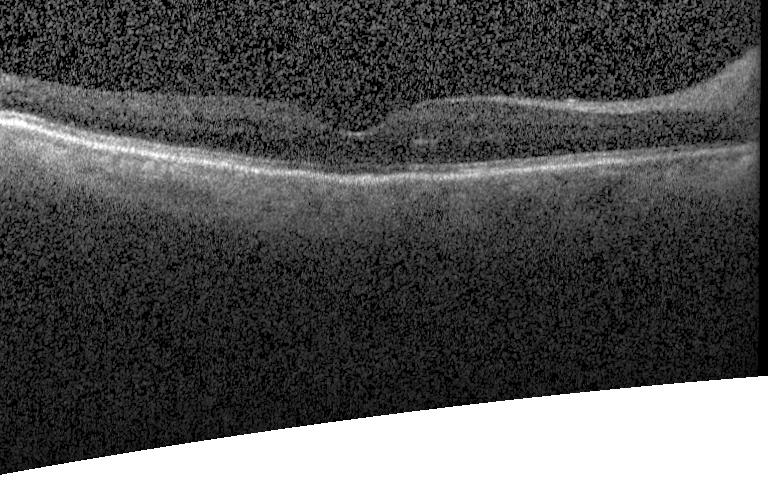
Spectral-domain optical coherence tomography · OCT B-scan.
This B-scan demonstrates neither choroidal neovascularization, diabetic macular edema, nor drusen.